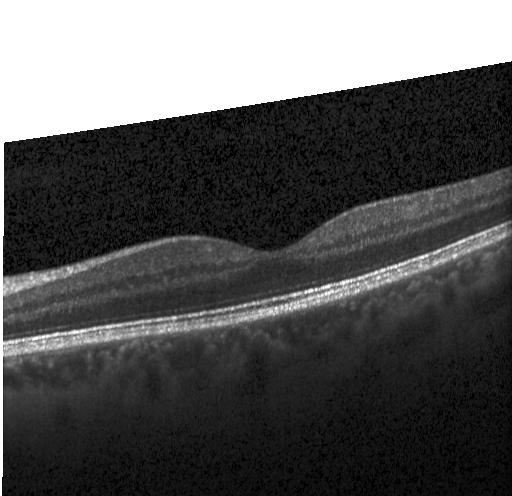 Finding: no evidence of choroidal neovascularization, diabetic macular edema, or drusen.